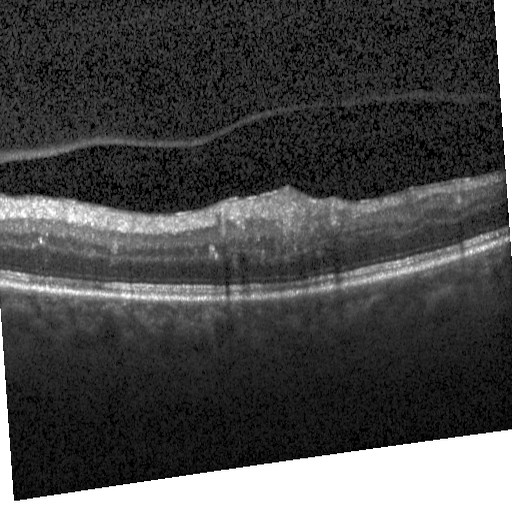

OCT scan showing diabetic macular edema.